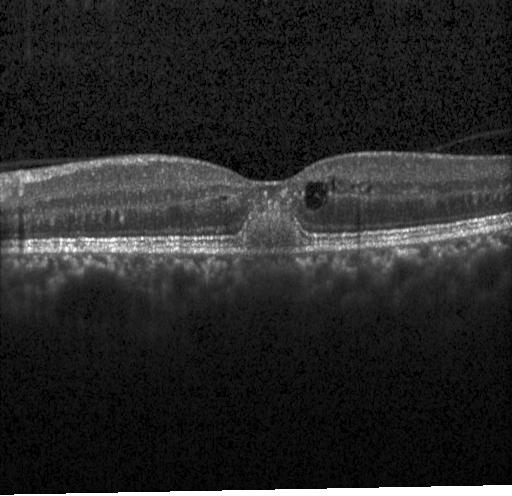 Spectral-domain optical coherence tomography, centered on the fovea, Heidelberg Spectralis, retinal OCT cross-section.
Finding: choroidal neovascularization.